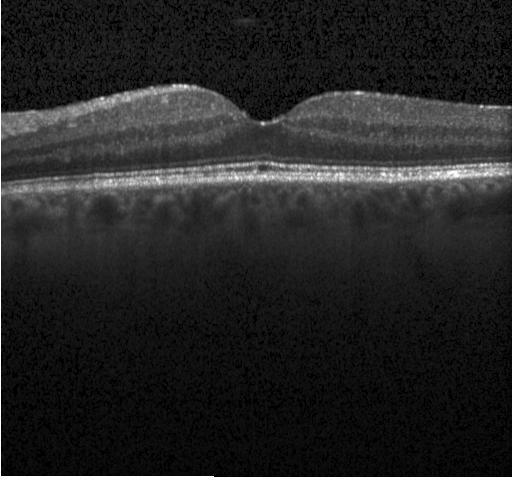 Spectral-domain OCT, Heidelberg Spectralis, OCT line scan. Assessment: no evidence of choroidal neovascularization, diabetic macular edema, or drusen.